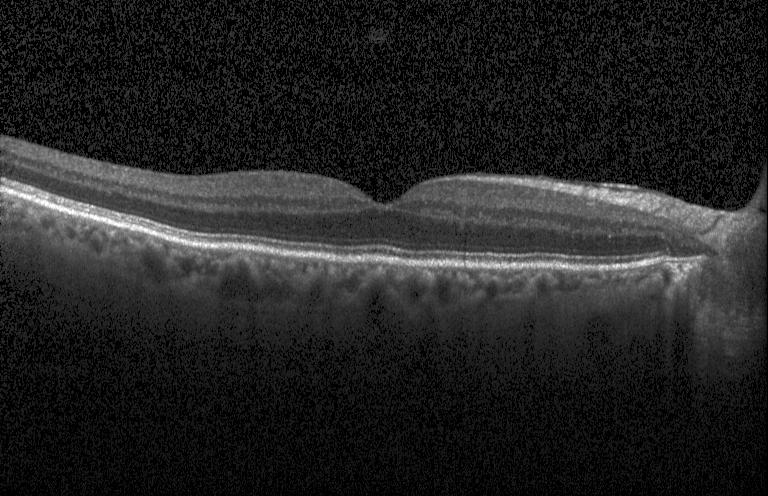
Acquired on a Heidelberg Spectralis, macular scan, SD-OCT, retinal OCT B-scan — Impression: neither CNV, DME, nor drusen.